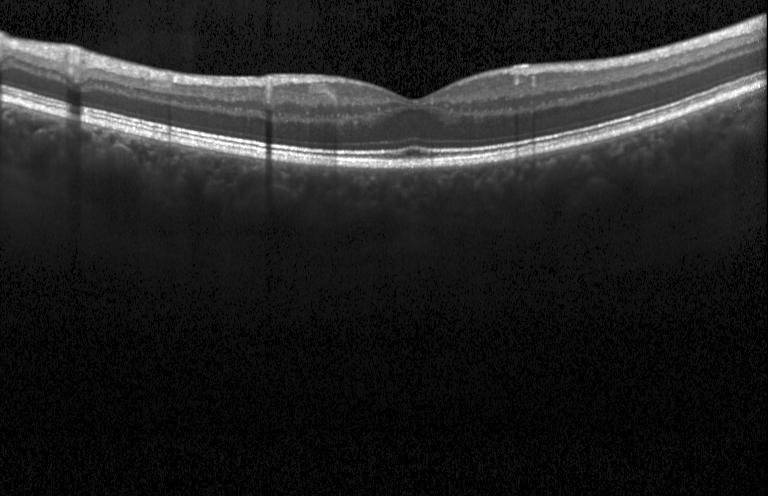 Macular OCT demonstrating neither choroidal neovascularization, diabetic macular edema, nor drusen.